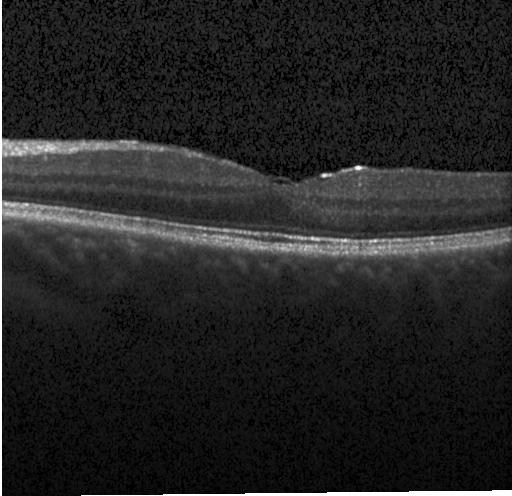
Retinal OCT B-scan. Spectral-domain optical coherence tomography. Neither choroidal neovascularization, diabetic macular edema, nor drusen.